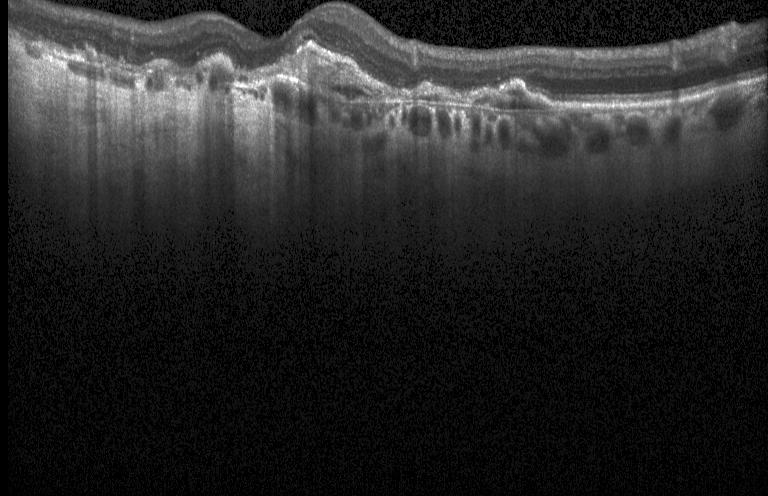
Macular OCT demonstrating CNV.